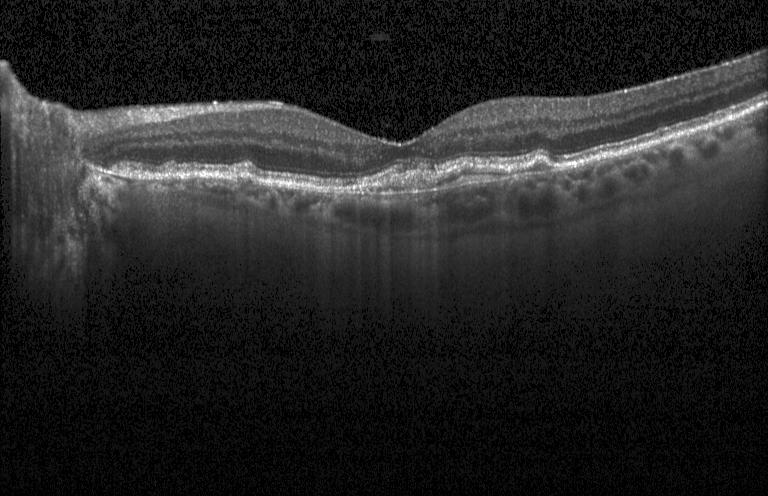

Retinal OCT cross-section showing a choroidal neovascular membrane.